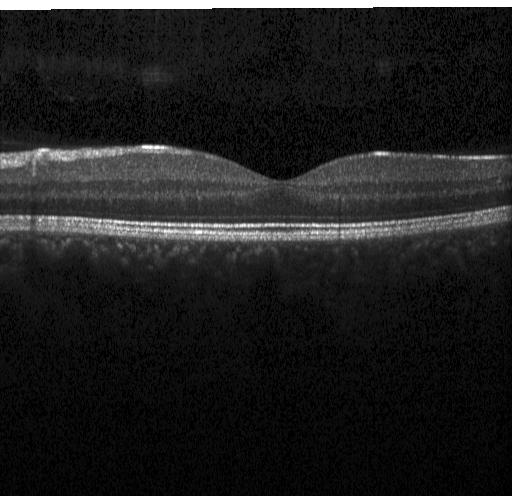 OCT B-scan — Macular OCT: no evidence of choroidal neovascularization, diabetic macular edema, or drusen.